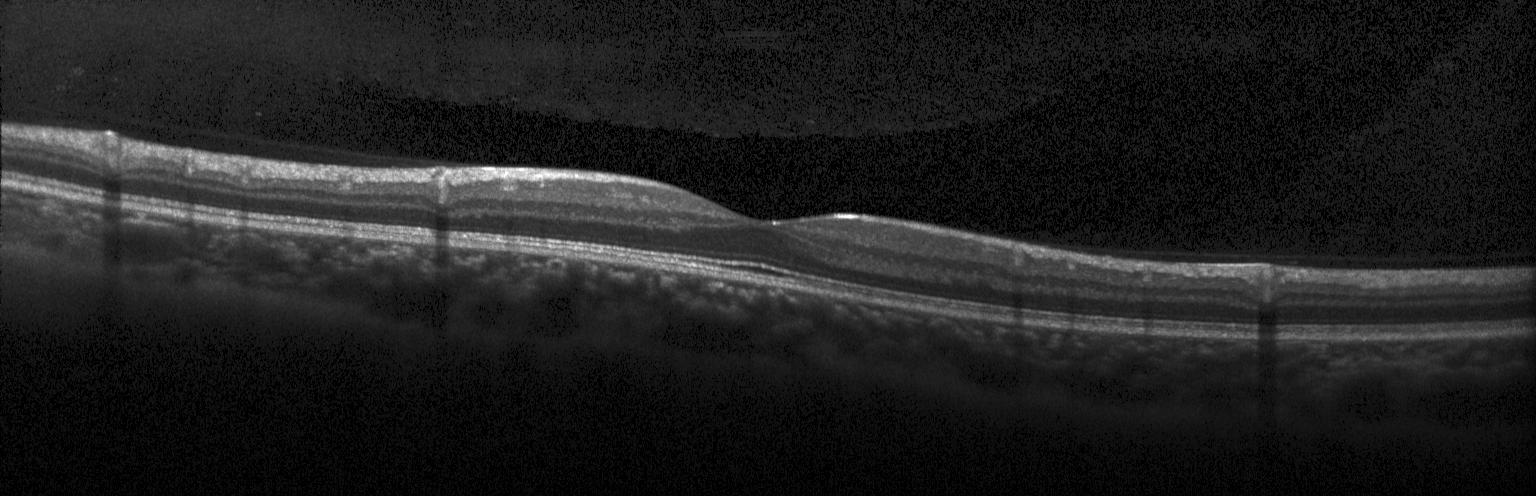
Spectral-domain optical coherence tomography · optical coherence tomography scan.
Dx: no CNV, no DME, and no drusen.